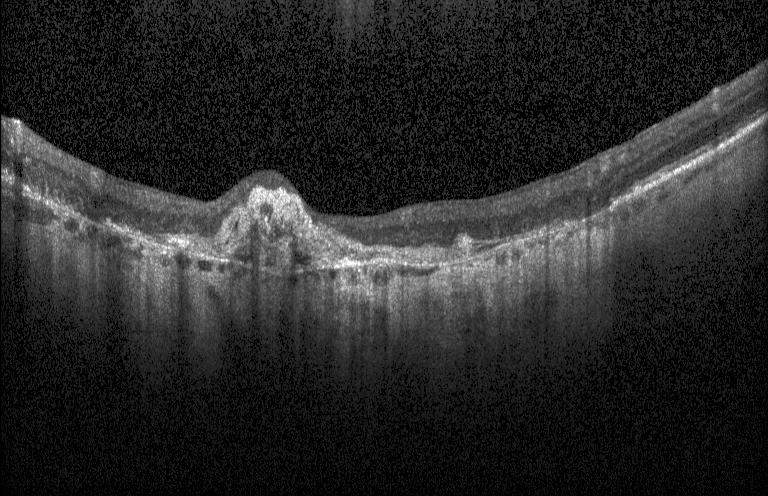
OCT line scan · acquired on a Heidelberg Spectralis — Diagnosis: CNV.